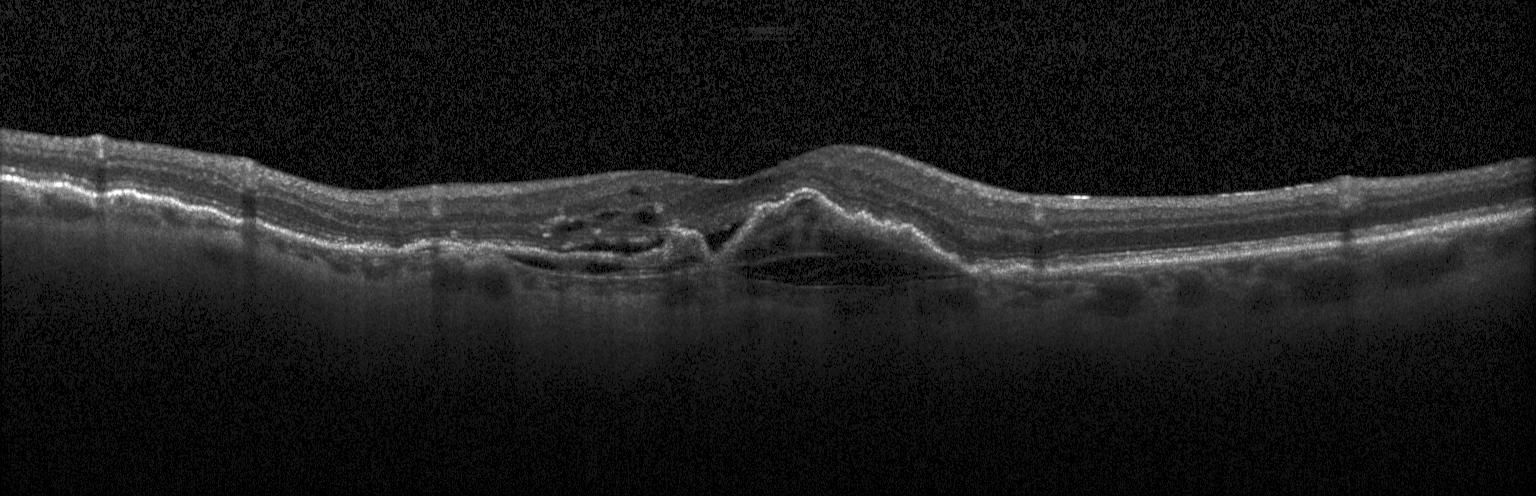
Diagnosis: a choroidal neovascular membrane.